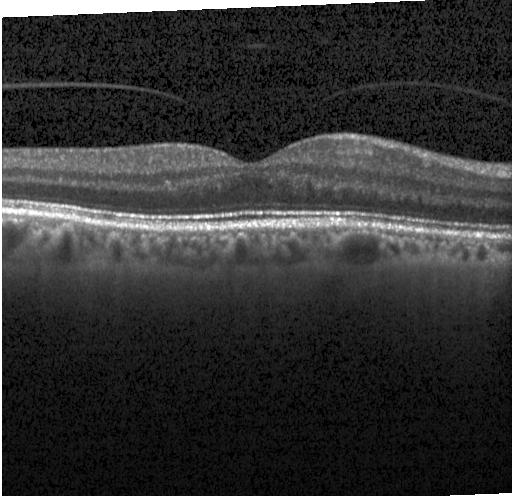 Retinal OCT B-scan, instrument: Heidelberg Spectralis, fovea-centered, spectral-domain OCT. No choroidal neovascularization, no diabetic macular edema, and no drusen.